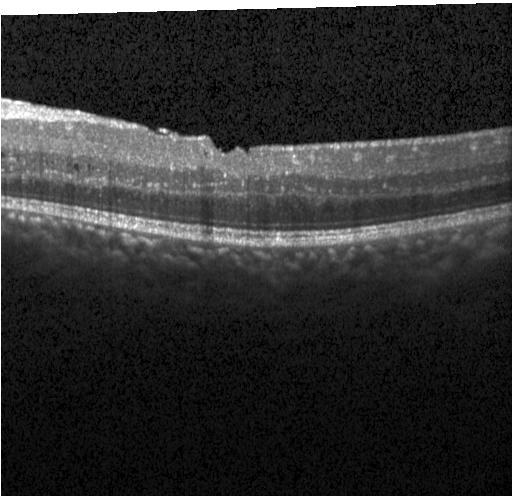

Macular OCT: diabetic macular edema.